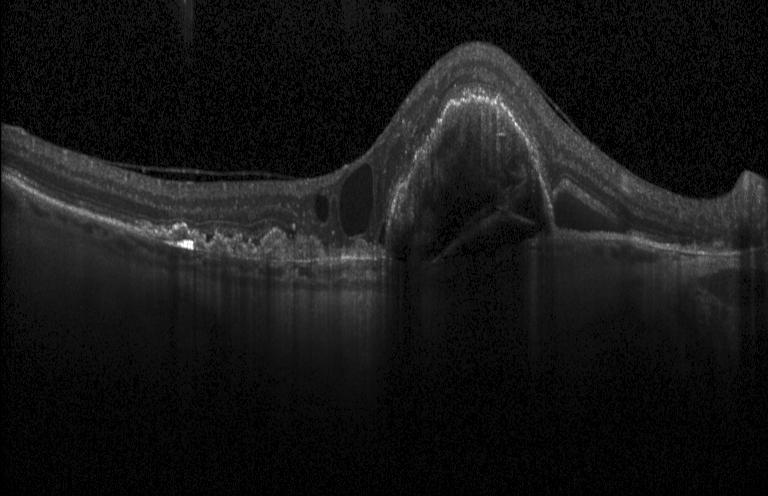 Optical coherence tomography B-scan.
Assessment: CNV.